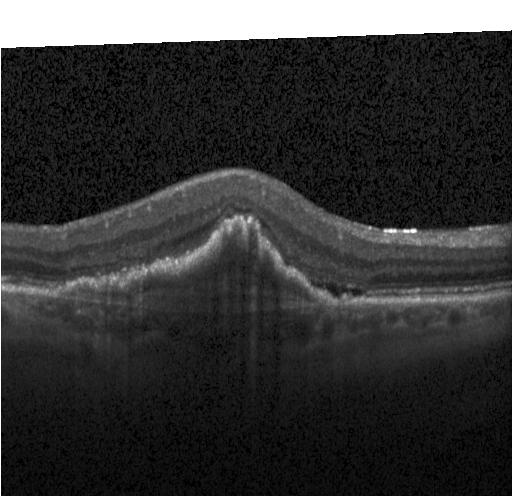 SD-OCT. Optical coherence tomography B-scan. Impression: choroidal neovascularization.